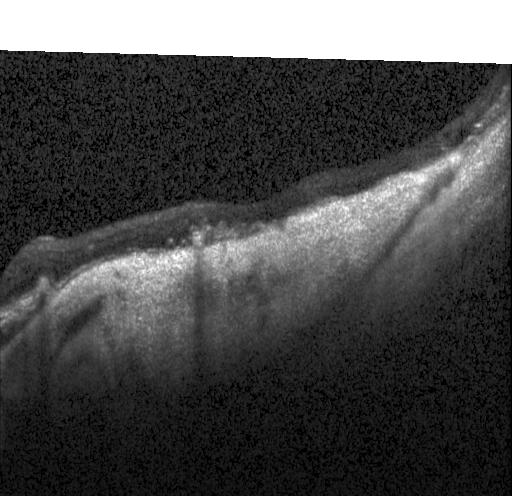
Diagnosis: CNV.